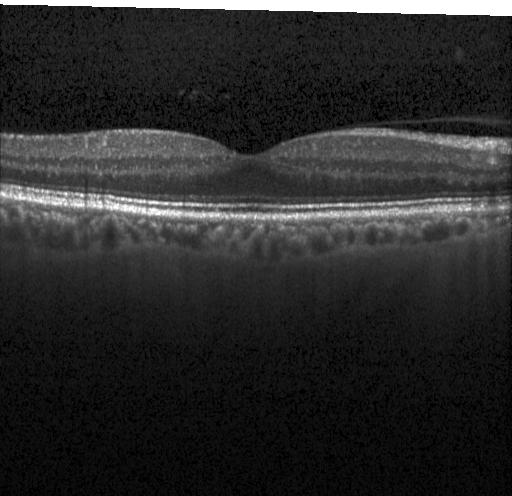

Impression: neither choroidal neovascularization, diabetic macular edema, nor drusen.